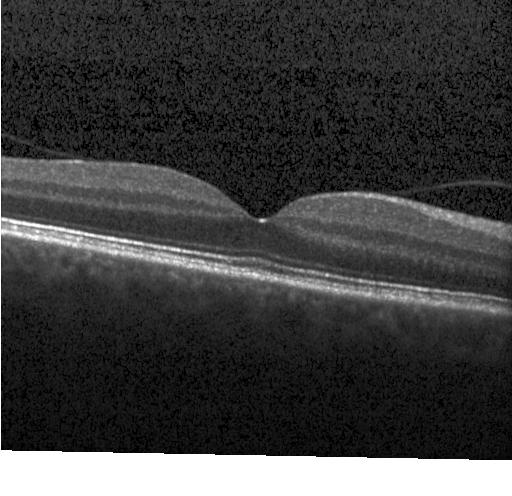 Optical coherence tomography scan. Heidelberg Spectralis OCT system — Finding: no choroidal neovascularization, diabetic macular edema, or drusen.